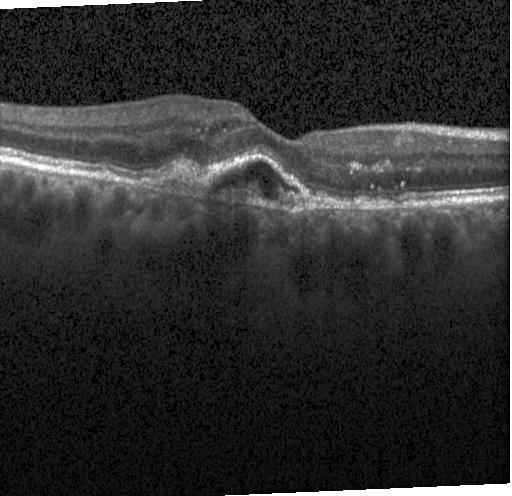

OCT B-scan.
Finding: a choroidal neovascular membrane.